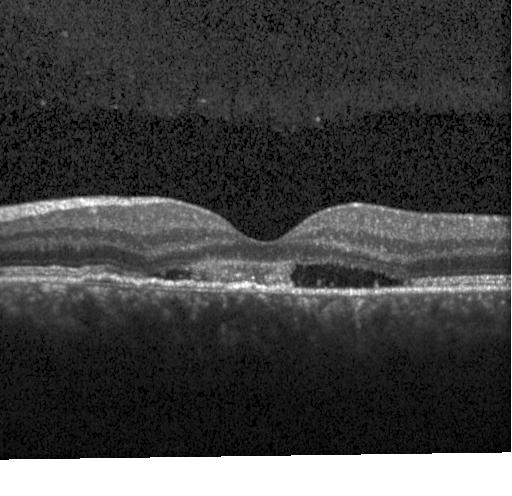
Optical coherence tomography B-scan. Finding: a choroidal neovascular membrane.